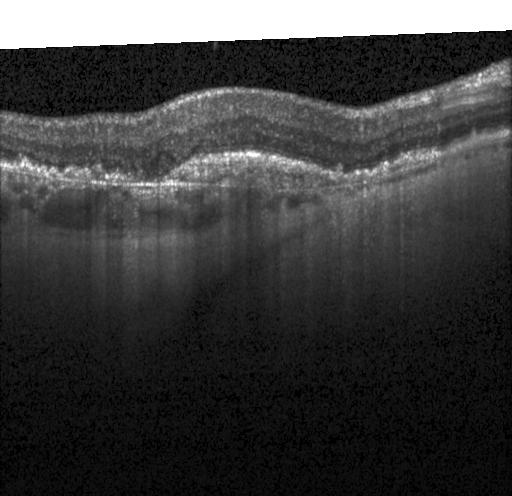
OCT line scan · instrument: Heidelberg Spectralis · macular scan. OCT finding: choroidal neovascularization.